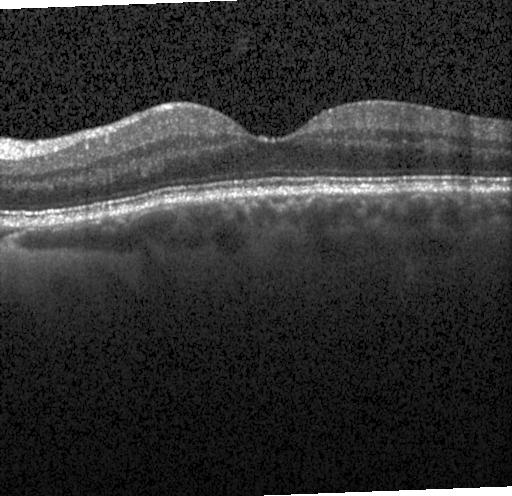

Heidelberg Spectralis OCT system; OCT line scan; spectral-domain OCT
This B-scan demonstrates no evidence of choroidal neovascularization, diabetic macular edema, or drusen.